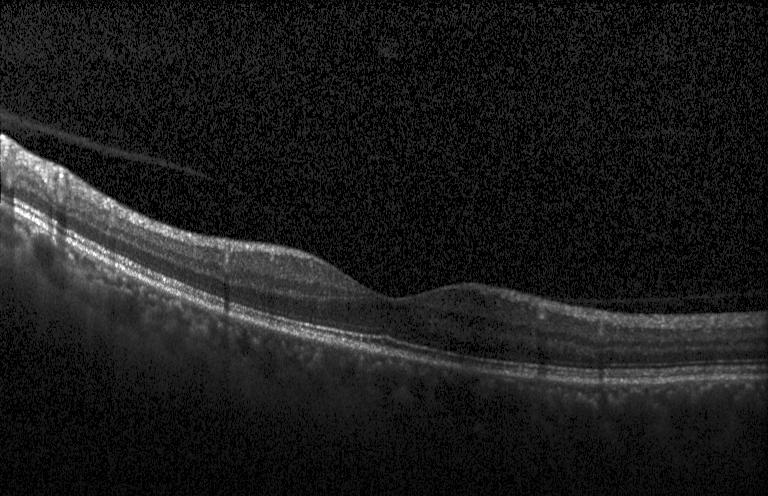

Centered on the fovea. Spectral-domain OCT. Optical coherence tomography B-scan. Instrument: Heidelberg Spectralis.
Finding: no choroidal neovascularization, diabetic macular edema, or drusen.